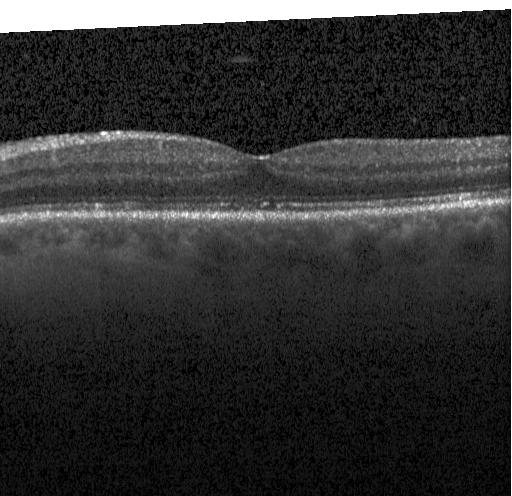 Diagnosis: no evidence of choroidal neovascularization, diabetic macular edema, or drusen.